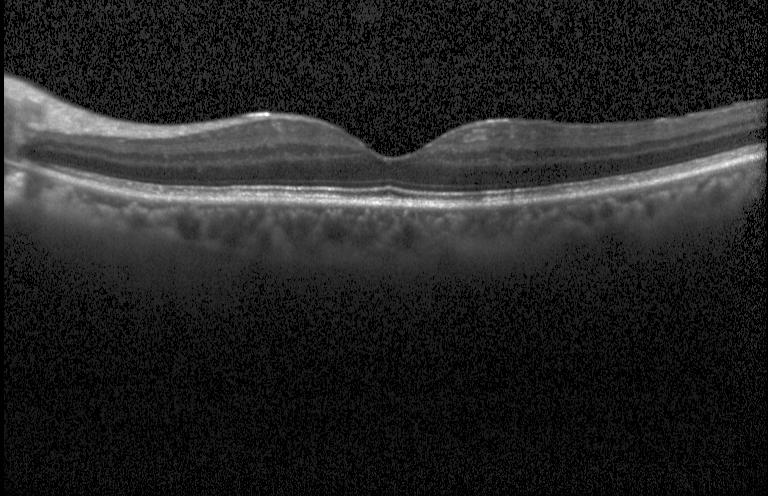
Horizontal scan through the fovea. Spectral-domain optical coherence tomography. Heidelberg Spectralis OCT system. Retinal OCT cross-section — Dx: neither choroidal neovascularization, diabetic macular edema, nor drusen.